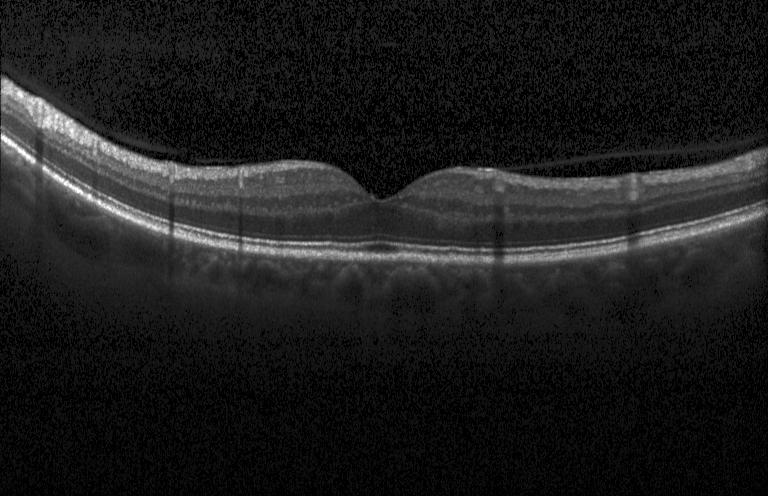

Horizontal scan through the fovea, spectral-domain optical coherence tomography, Heidelberg Spectralis OCT system, optical coherence tomography B-scan
Impression: no choroidal neovascularization, no diabetic macular edema, and no drusen.